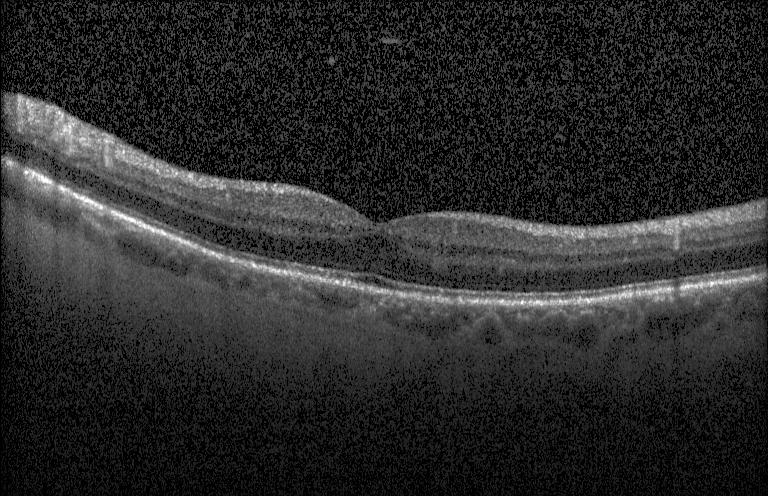

Macular scan · optical coherence tomography scan.
Diagnosis: no evidence of choroidal neovascularization, diabetic macular edema, or drusen.